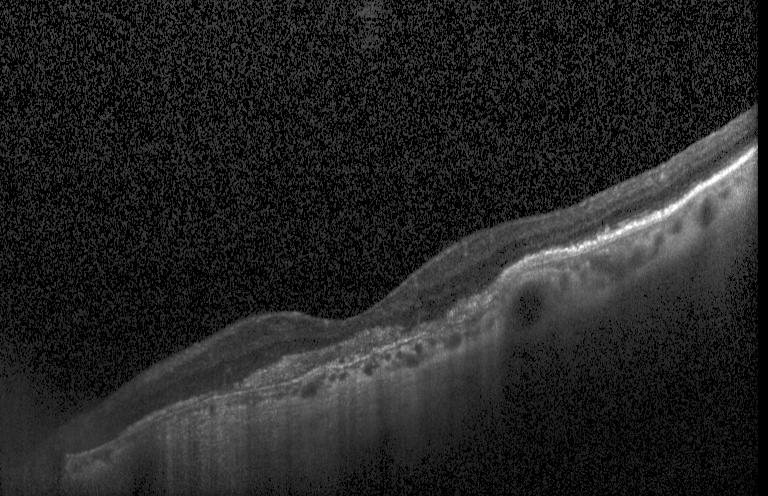 Optical coherence tomography scan; acquired on a Heidelberg Spectralis.
Assessment: a choroidal neovascular membrane.